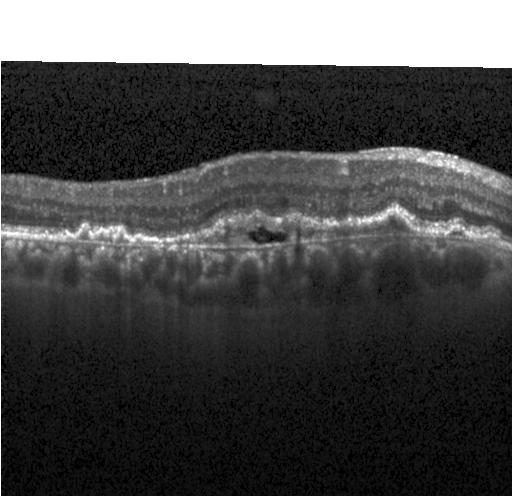
Macular OCT: CNV.